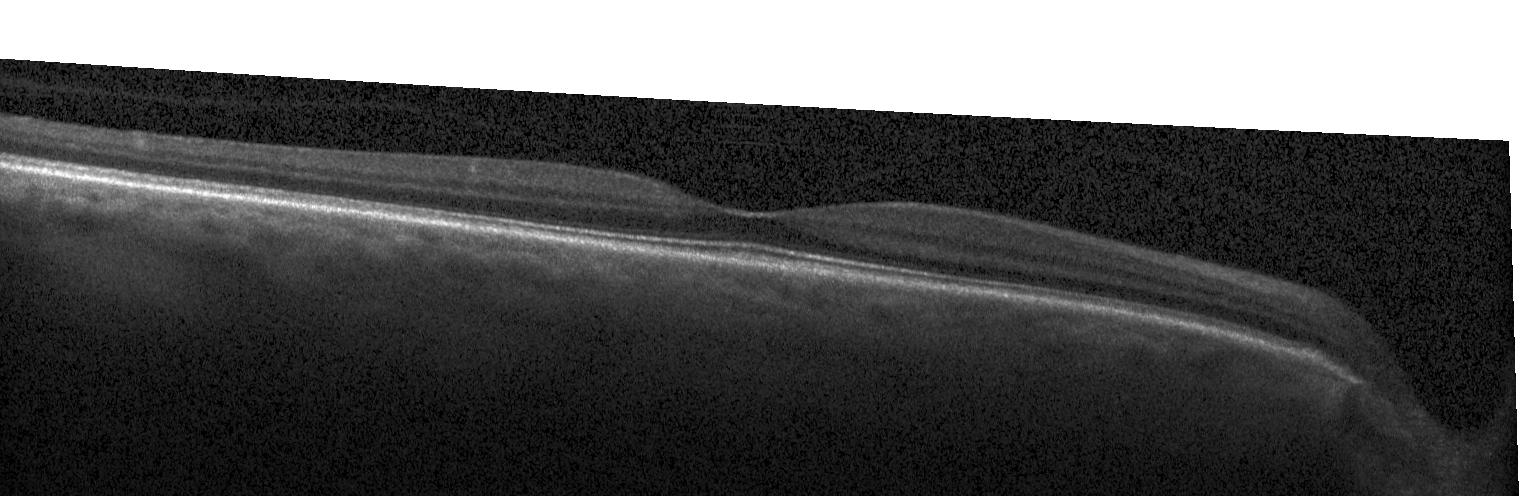
Macular OCT: no choroidal neovascularization, no diabetic macular edema, and no drusen.